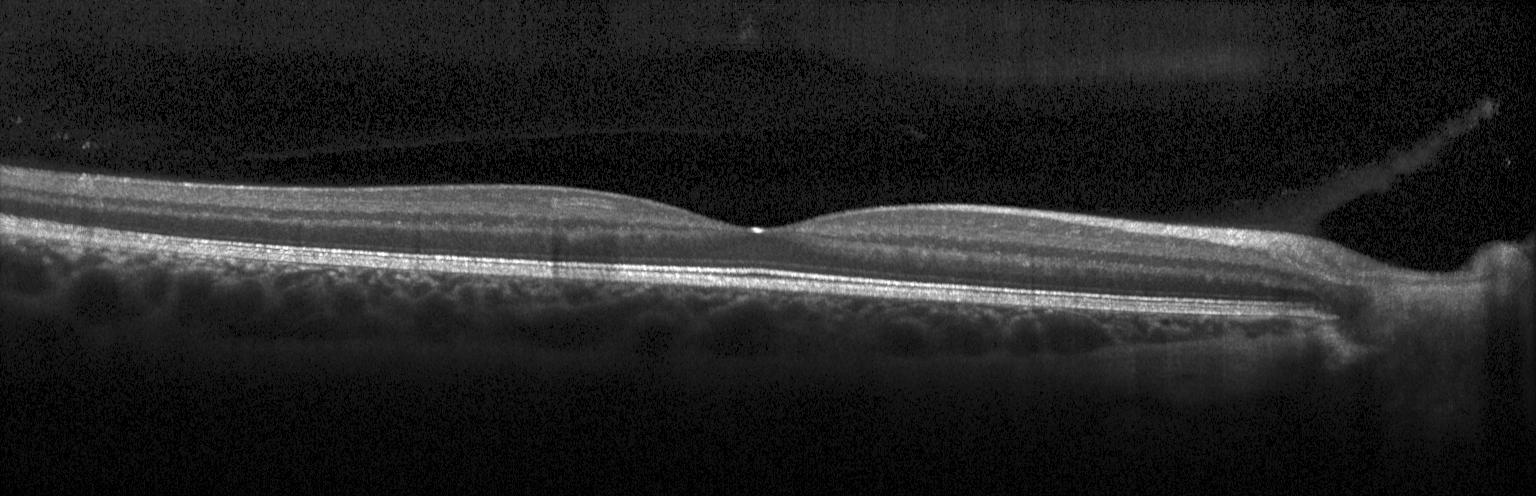
Heidelberg Spectralis, optical coherence tomography B-scan
Macular OCT: no CNV, no DME, and no drusen.